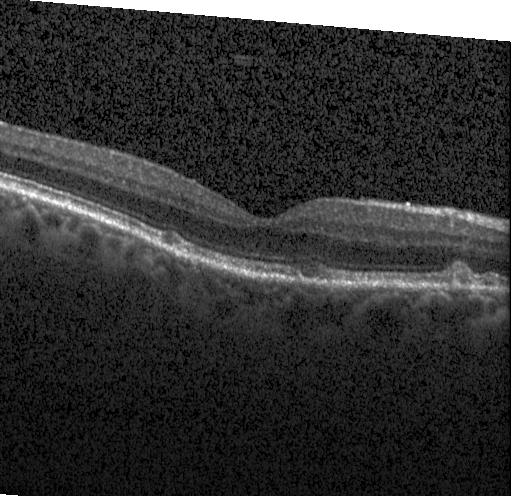

Heidelberg Spectralis, SD-OCT, OCT B-scan, horizontal scan through the fovea. Assessment: sub-RPE drusenoid deposits.